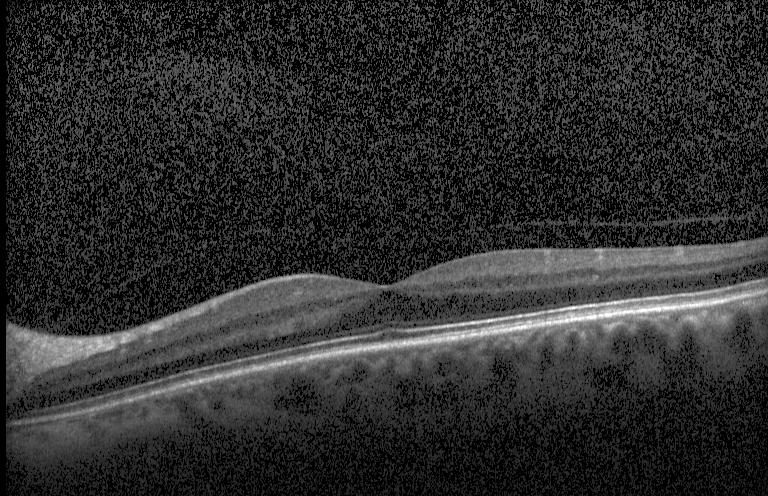
Retinal OCT B-scan — OCT finding: no CNV, DME, or drusen.